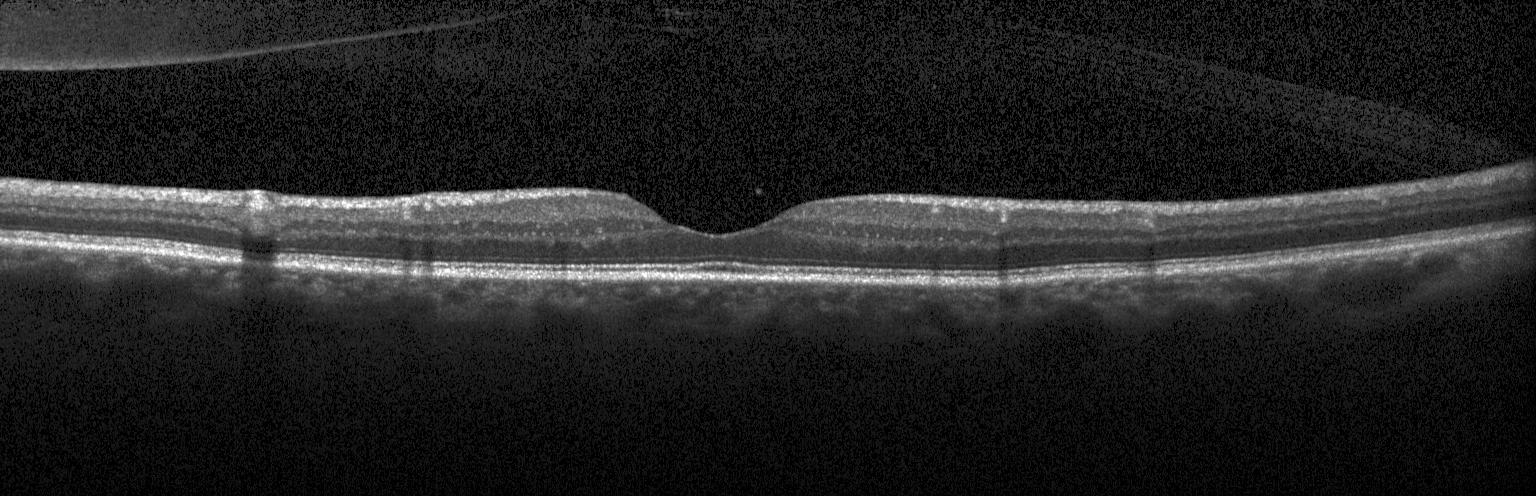 Retinal OCT B-scan · SD-OCT · through the macula
Diagnosis: neither choroidal neovascularization, diabetic macular edema, nor drusen.